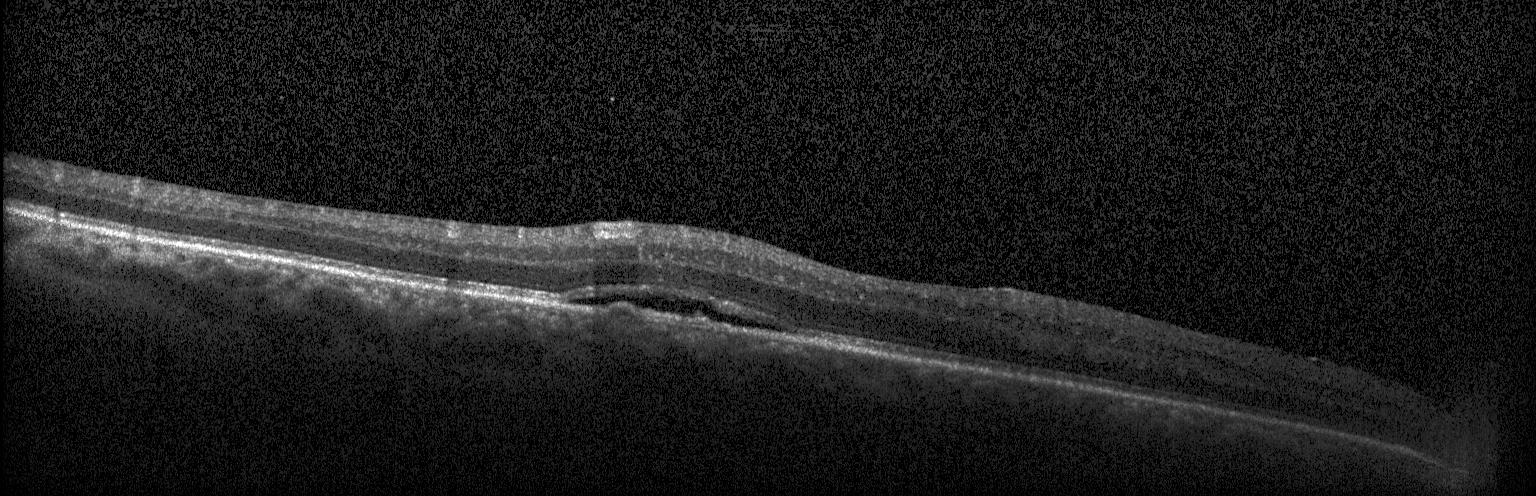
Heidelberg Spectralis · optical coherence tomography B-scan — Macular OCT: choroidal neovascularization (CNV).